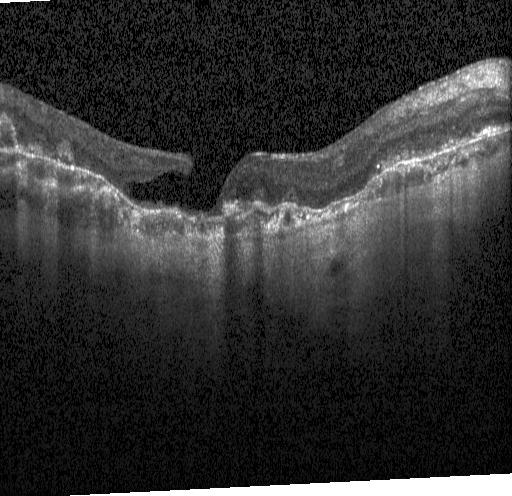
Macular OCT: a choroidal neovascular membrane.